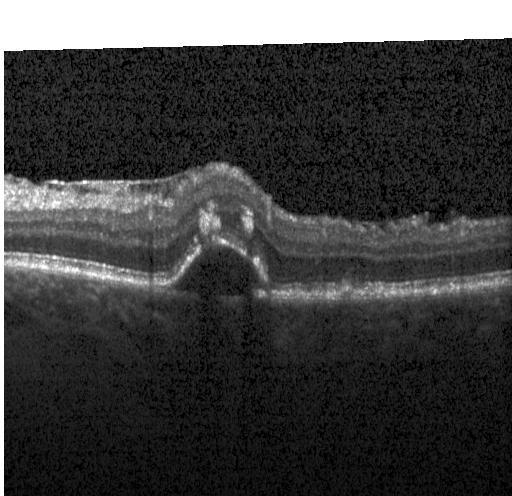 SD-OCT; OCT B-scan; horizontal scan through the fovea; acquired on a Heidelberg Spectralis. Finding: choroidal neovascularization (CNV).